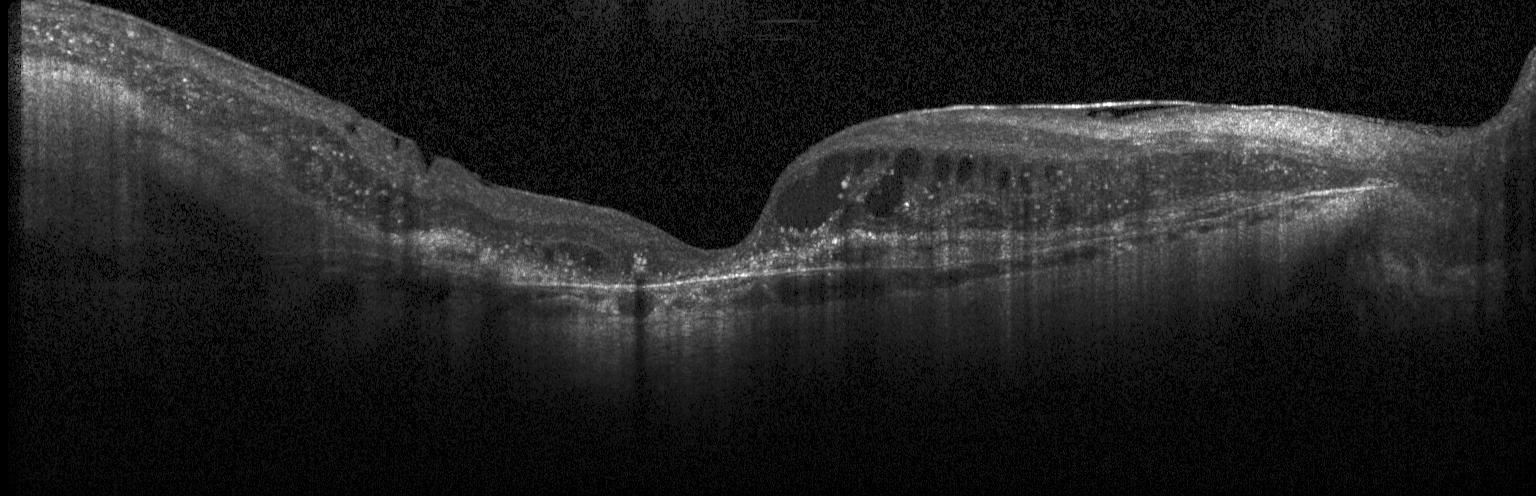

Heidelberg Spectralis; OCT B-scan; spectral-domain optical coherence tomography; centered on the fovea — A choroidal neovascular membrane.